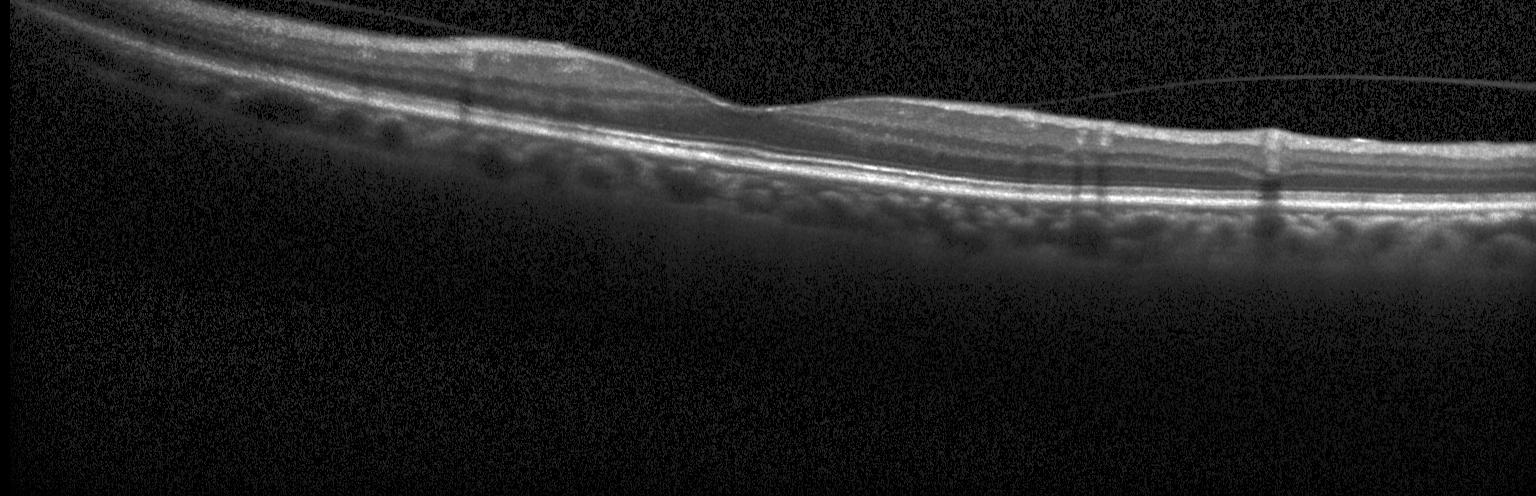 Optical coherence tomography scan. Spectral-domain OCT. Horizontal scan through the fovea — OCT finding: no CNV, DME, or drusen.